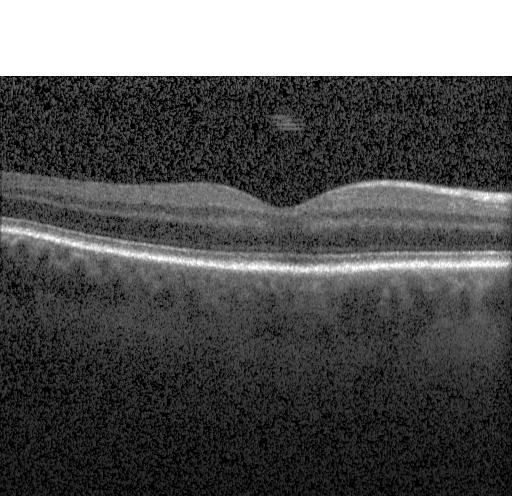 SD-OCT · OCT B-scan · acquired on a Heidelberg Spectralis. Impression: neither choroidal neovascularization, diabetic macular edema, nor drusen.